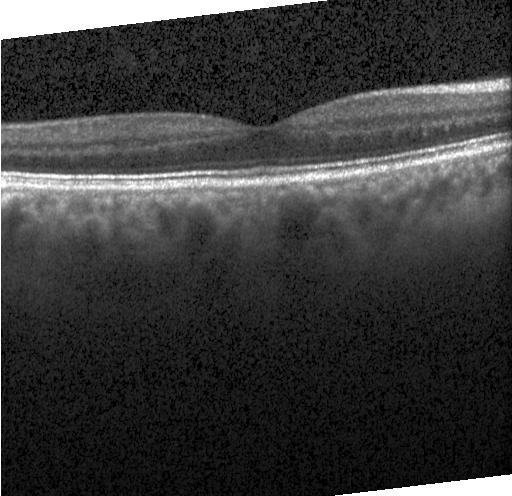

Impression: no evidence of CNV, DME, or drusen.